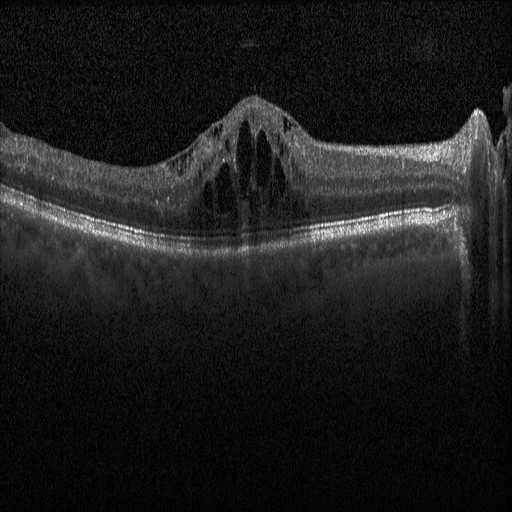 SD-OCT. Heidelberg Spectralis. Retinal OCT B-scan
Diabetic macular edema (DME).